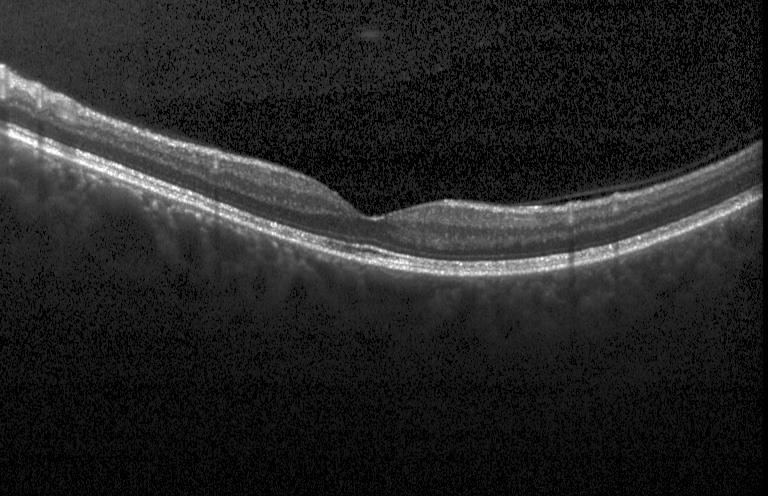

Fovea-centered; OCT B-scan; SD-OCT; acquired on a Heidelberg Spectralis.
Assessment: no CNV, DME, or drusen.